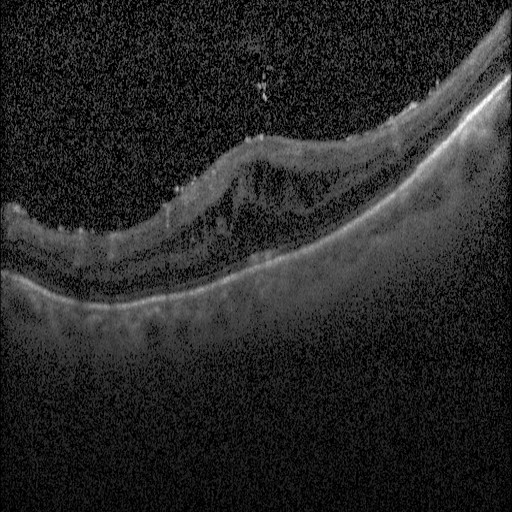

Spectral-domain OCT, optical coherence tomography scan, Heidelberg Spectralis OCT system, horizontal scan through the fovea
Dx: DME.